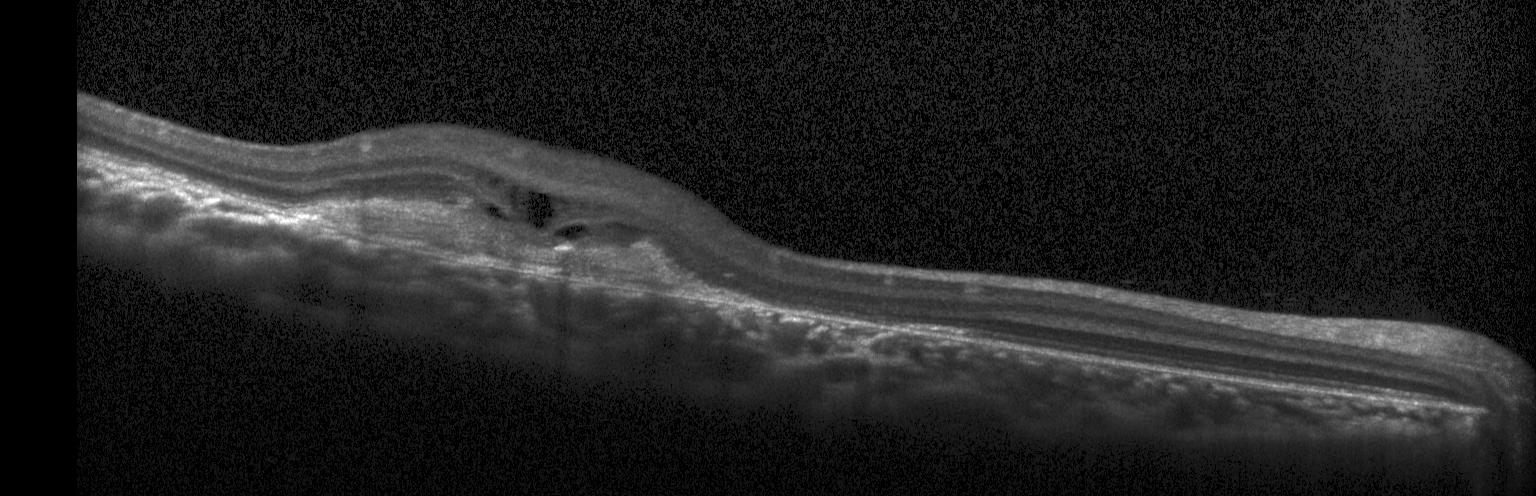

Heidelberg Spectralis · optical coherence tomography scan · spectral-domain OCT
This B-scan demonstrates choroidal neovascularization (CNV).